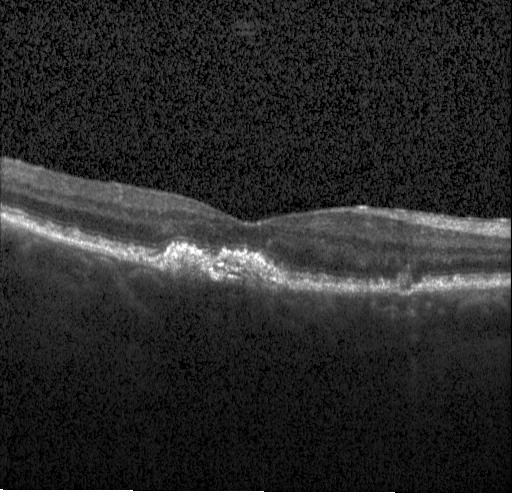

Optical coherence tomography B-scan. Finding: a choroidal neovascular membrane.